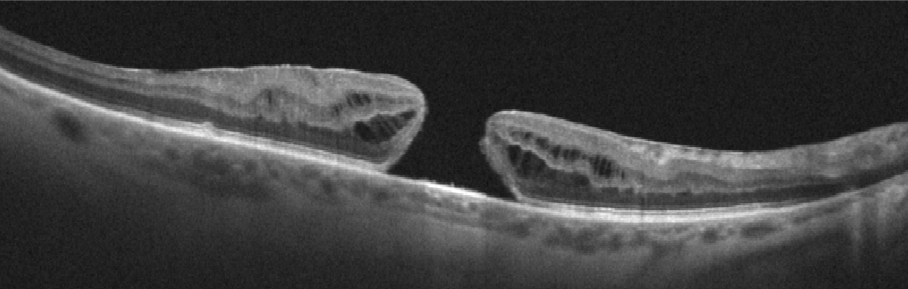
This B-scan demonstrates vitreomacular interface disease.